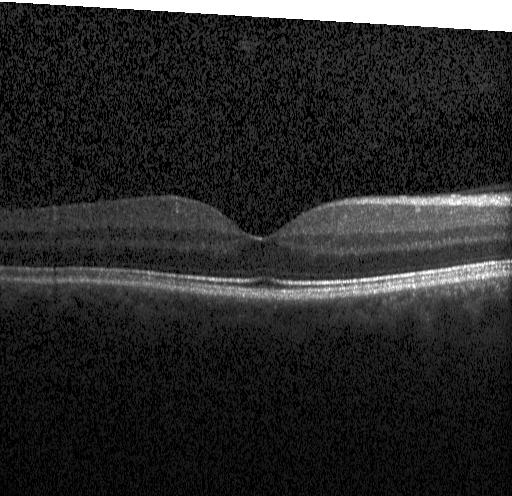 Instrument: Heidelberg Spectralis. Horizontal scan through the fovea. Retinal OCT cross-section.
OCT finding: neither CNV, DME, nor drusen.